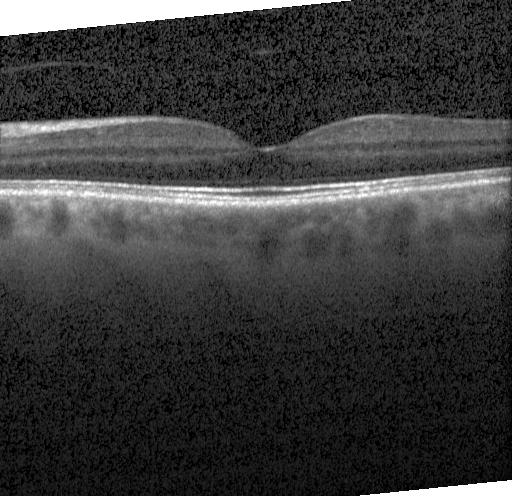

Finding: no choroidal neovascularization, no diabetic macular edema, and no drusen.